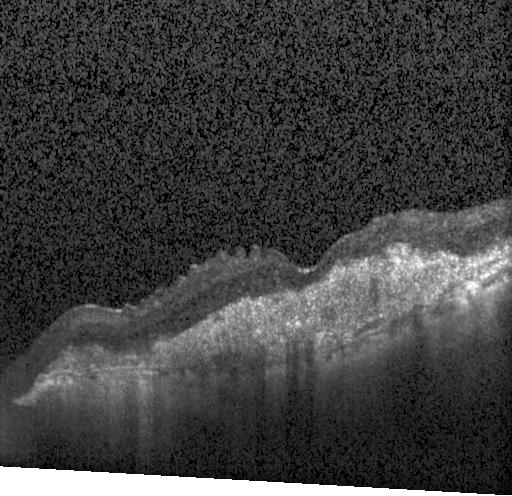
SD-OCT, fovea-centered, OCT line scan, instrument: Heidelberg Spectralis. Macular OCT: a choroidal neovascular membrane.